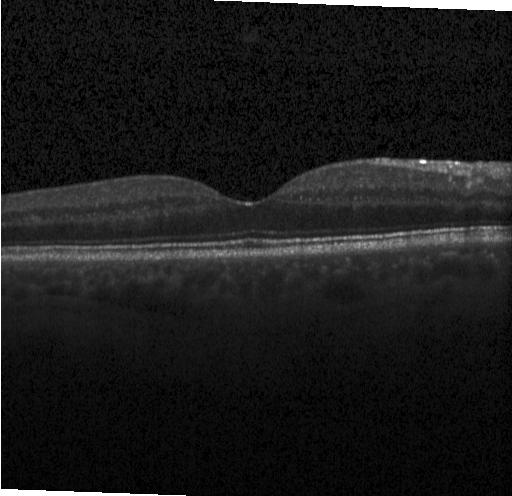
Retinal OCT cross-section; macular scan
Impression: no evidence of choroidal neovascularization, diabetic macular edema, or drusen.